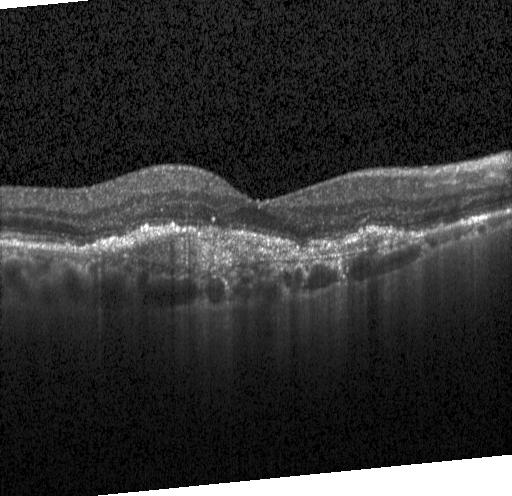

Finding: choroidal neovascularization (CNV).